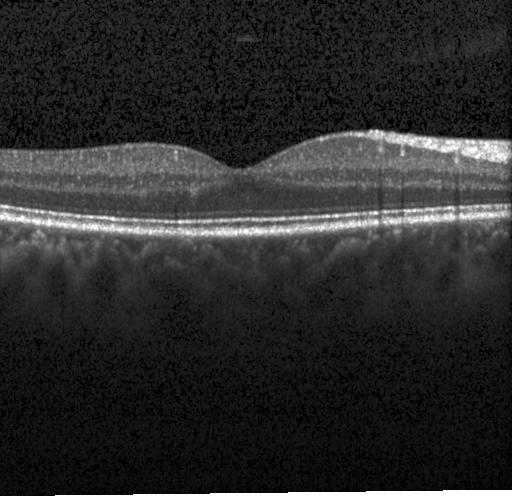

OCT line scan
The scan shows neither choroidal neovascularization, diabetic macular edema, nor drusen.